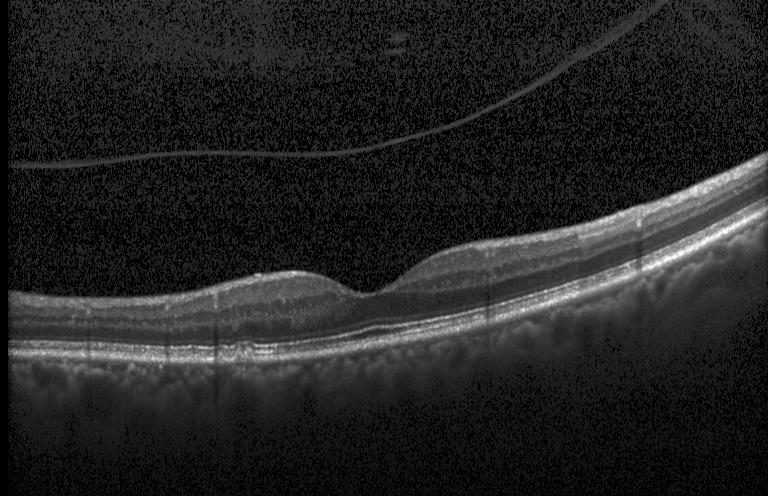

Acquired on a Heidelberg Spectralis. Fovea-centered. OCT B-scan — Finding: drusen.